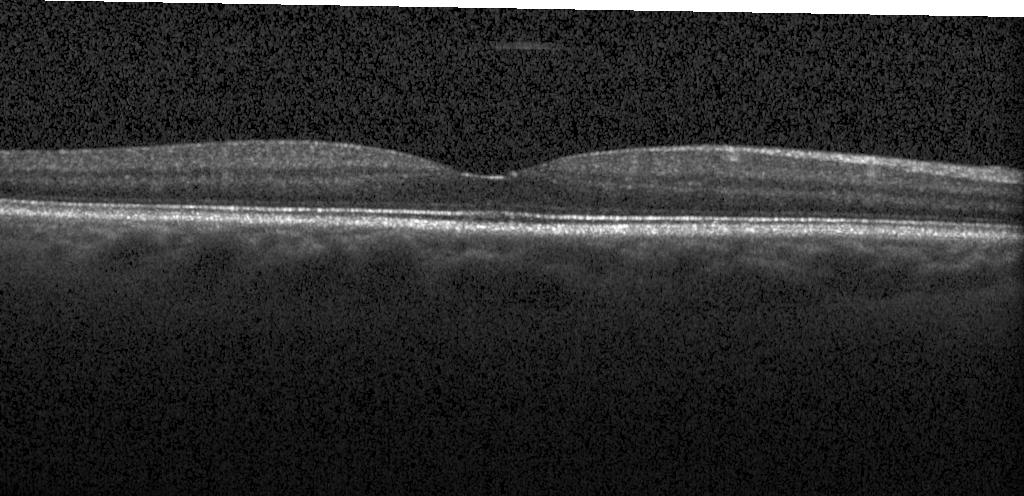 Fovea-centered, OCT B-scan.
Impression: no choroidal neovascularization, diabetic macular edema, or drusen.